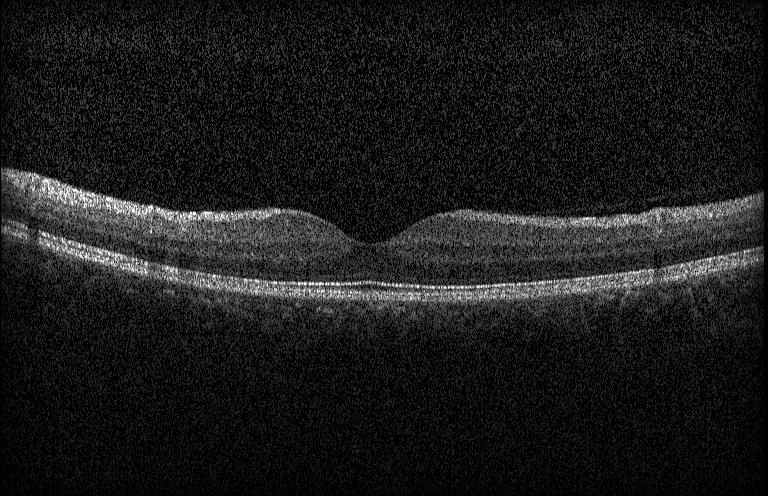

OCT line scan.
Diagnosis: no choroidal neovascularization, no diabetic macular edema, and no drusen.